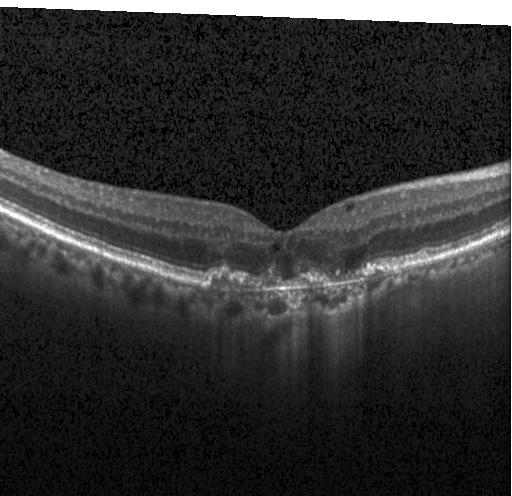
CNV.